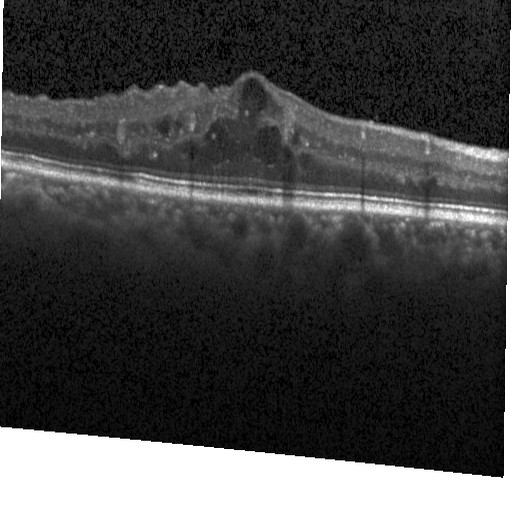
Diagnosis: diabetic macular edema.